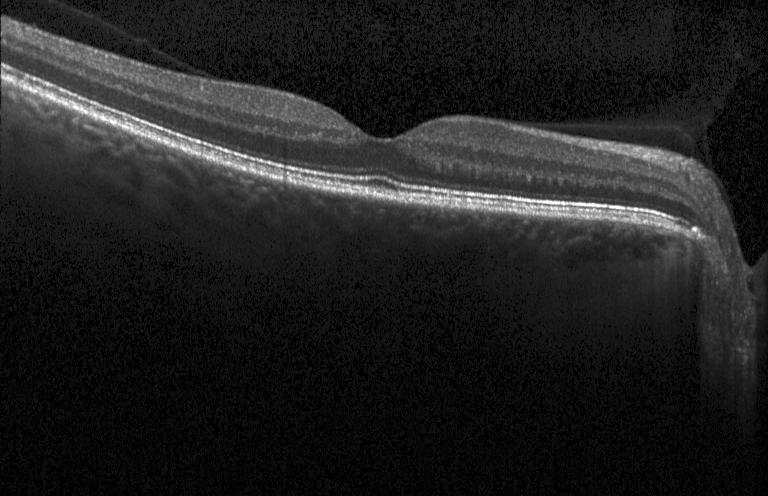

Optical coherence tomography B-scan
This B-scan demonstrates no evidence of choroidal neovascularization, diabetic macular edema, or drusen.